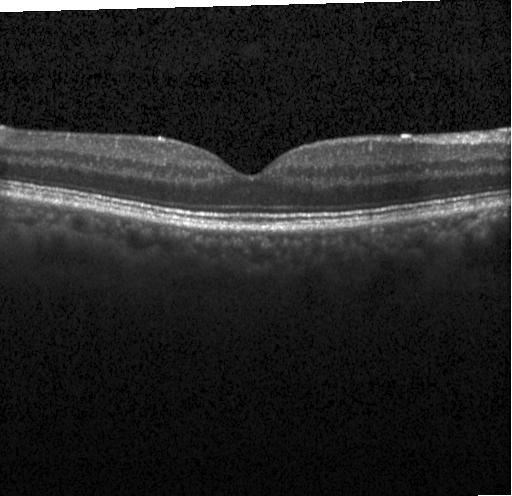

Optical coherence tomography scan, centered on the fovea, acquired on a Heidelberg Spectralis, spectral-domain OCT — No choroidal neovascularization, no diabetic macular edema, and no drusen.